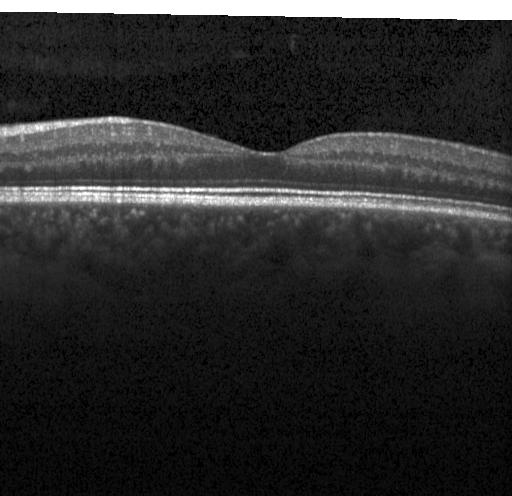

Impression: no evidence of choroidal neovascularization, diabetic macular edema, or drusen.